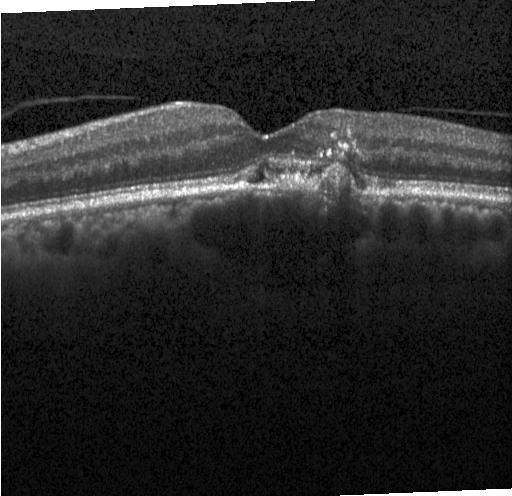 Horizontal scan through the fovea. Acquired on a Heidelberg Spectralis. SD-OCT. Retinal OCT B-scan — Diagnosis: a choroidal neovascular membrane.